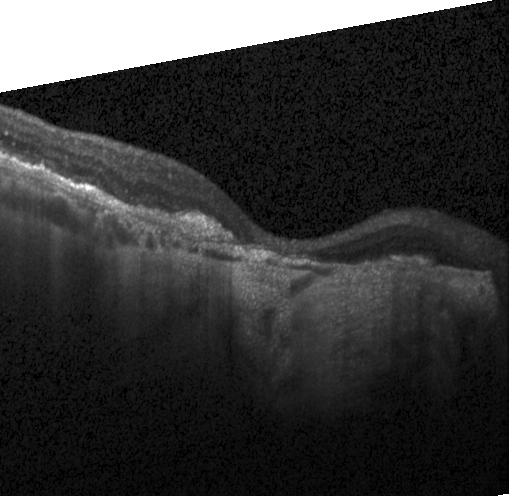

OCT line scan. Through the macula. Heidelberg Spectralis OCT system — Finding: choroidal neovascularization (CNV).